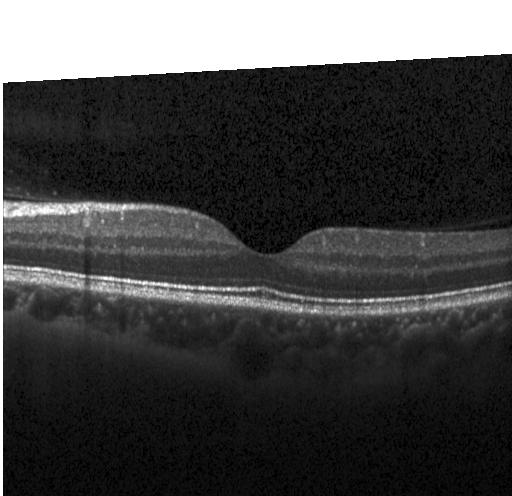
Assessment: no choroidal neovascularization, diabetic macular edema, or drusen.